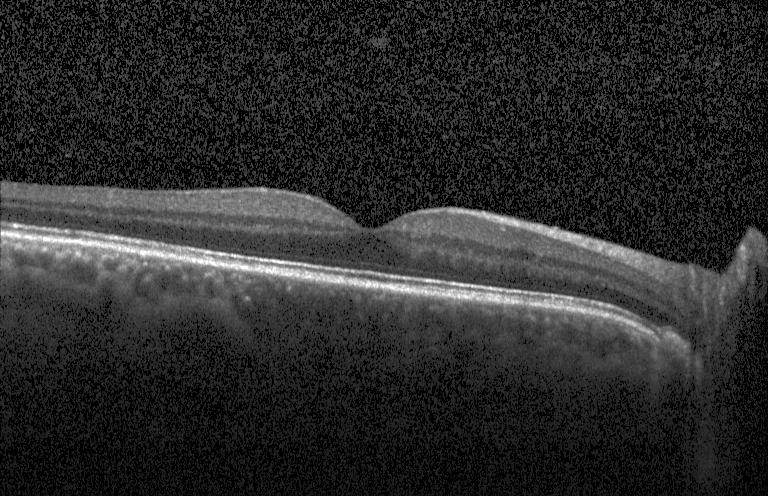 Optical coherence tomography B-scan — OCT finding: no choroidal neovascularization, diabetic macular edema, or drusen.